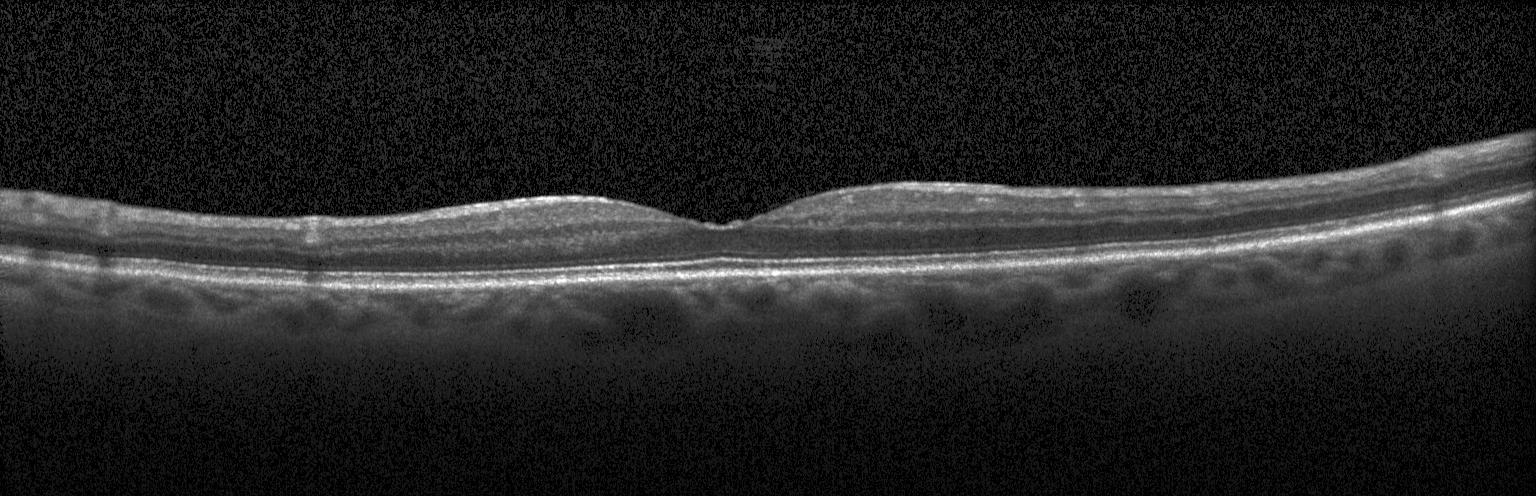
OCT finding: neither CNV, DME, nor drusen.